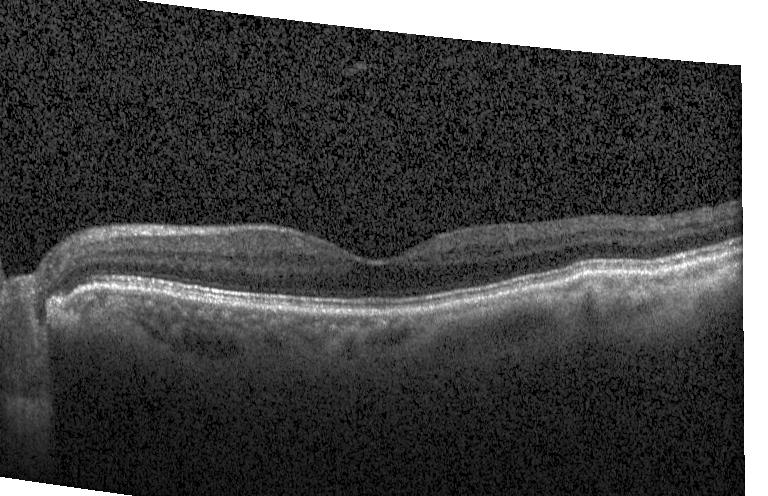 The scan shows no choroidal neovascularization, diabetic macular edema, or drusen.